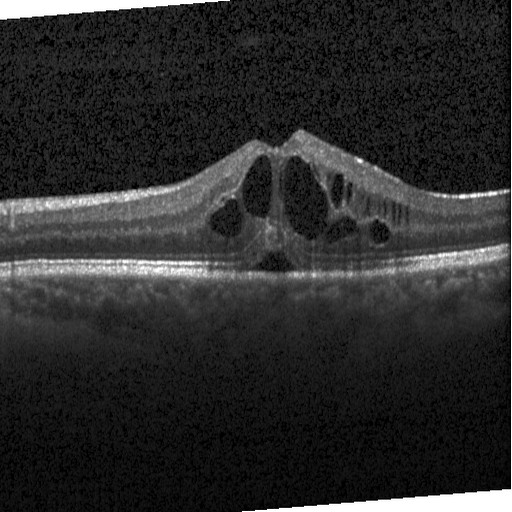 Heidelberg Spectralis; OCT B-scan; SD-OCT.
Diagnosis: diabetic macular edema (DME).